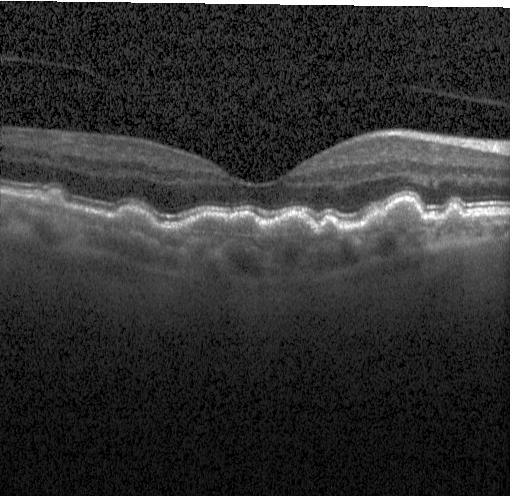

Retinal OCT cross-section. SD-OCT. Instrument: Heidelberg Spectralis. Dx: multiple drusen.